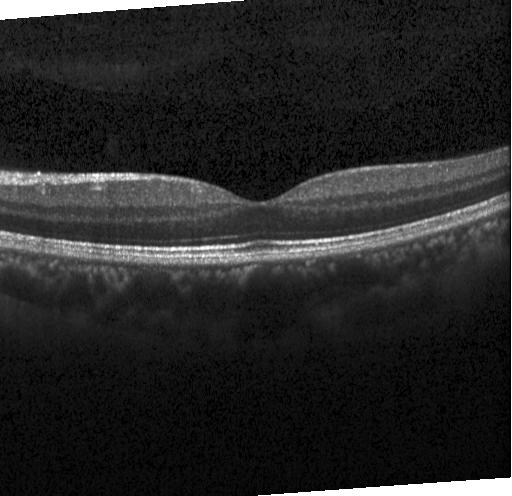
OCT scan showing no CNV, DME, or drusen.